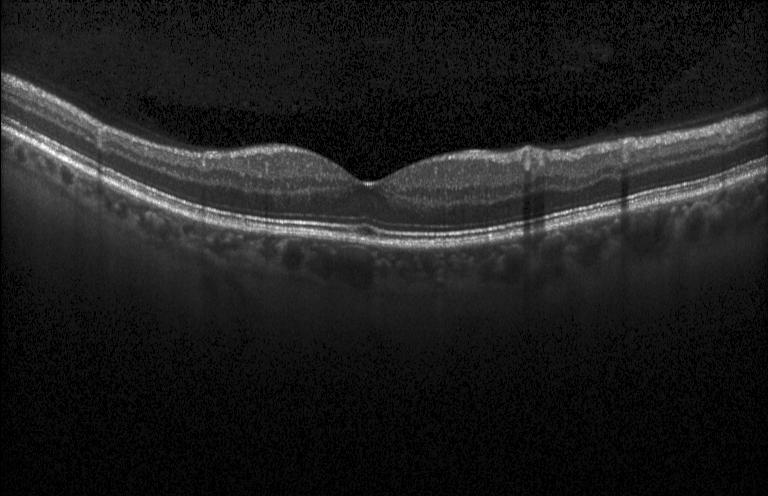

Through the macula · retinal OCT B-scan
Impression: neither CNV, DME, nor drusen.